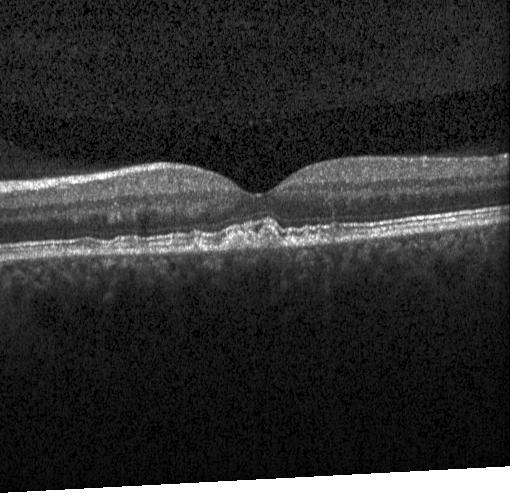 Through the macula; spectral-domain OCT; OCT line scan — The scan shows multiple drusen.